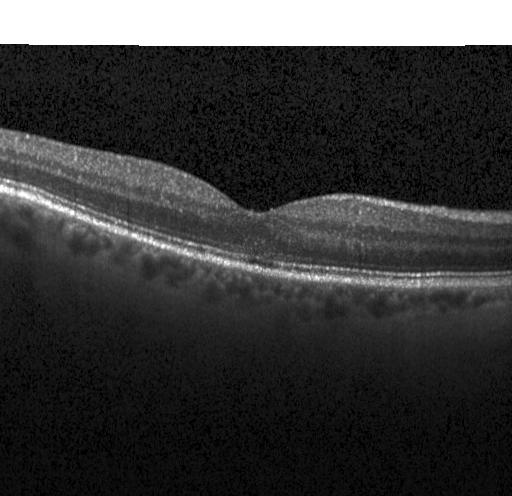 OCT finding: no CNV, no DME, and no drusen.